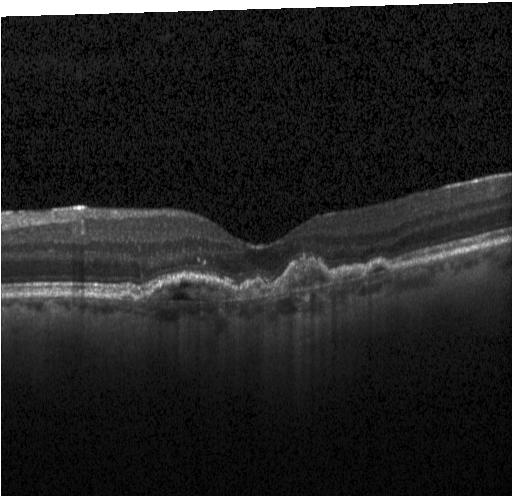

OCT B-scan — This B-scan demonstrates a choroidal neovascular membrane.